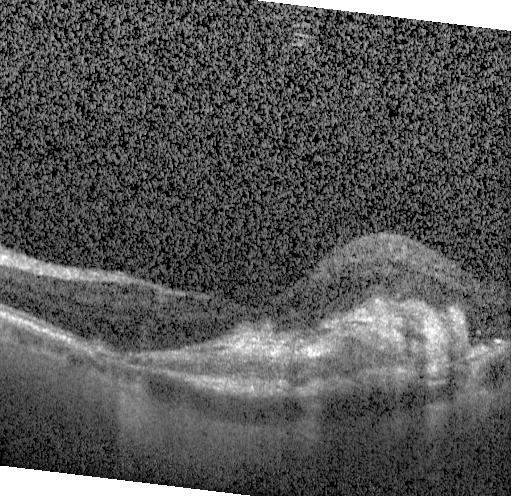

Through the macula; optical coherence tomography B-scan — Impression: choroidal neovascularization (CNV).